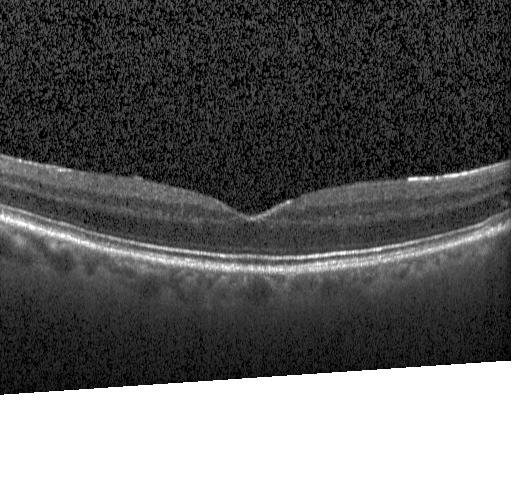

Finding: no evidence of choroidal neovascularization, diabetic macular edema, or drusen.